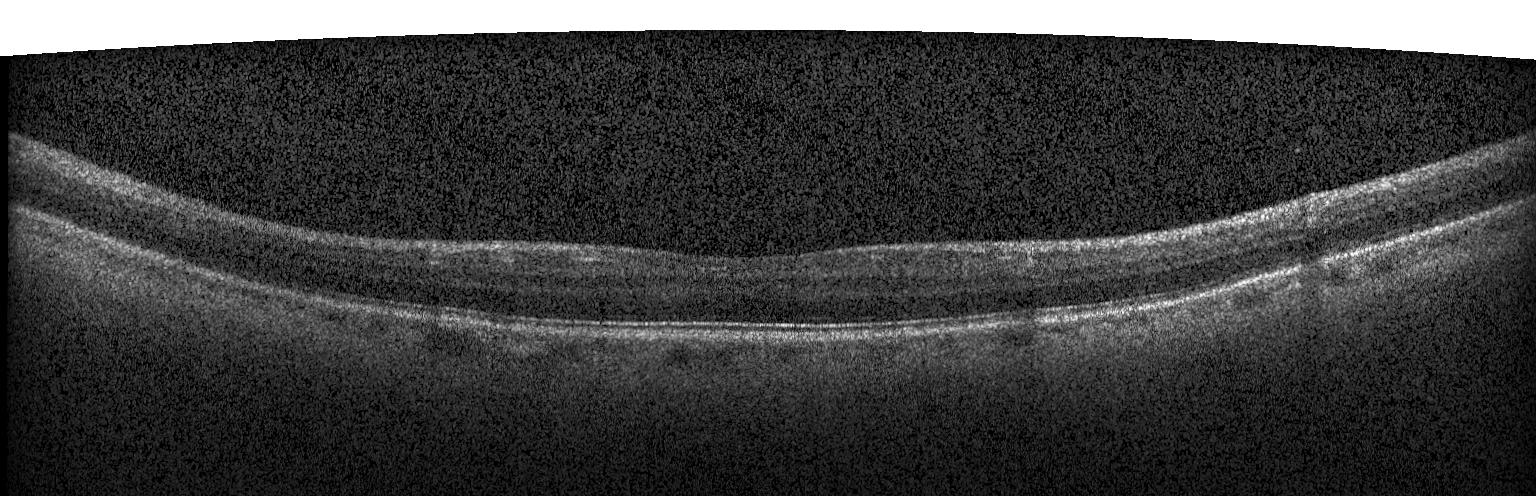 Retinal OCT B-scan.
The scan shows no CNV, DME, or drusen.